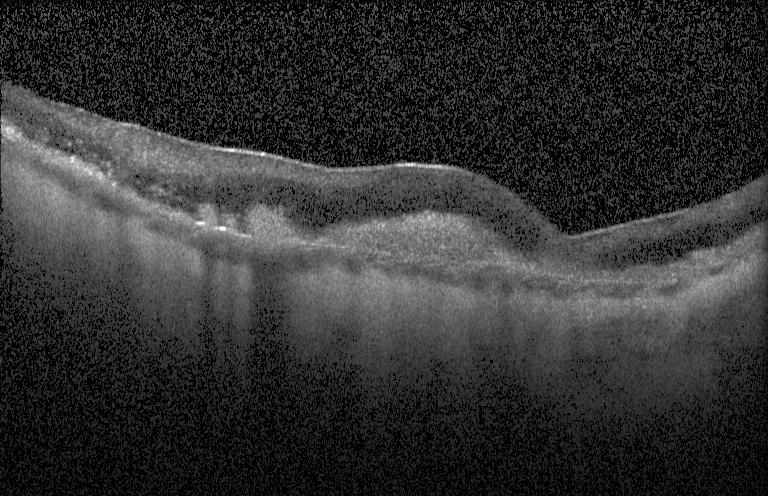 Diagnosis: choroidal neovascularization (CNV).